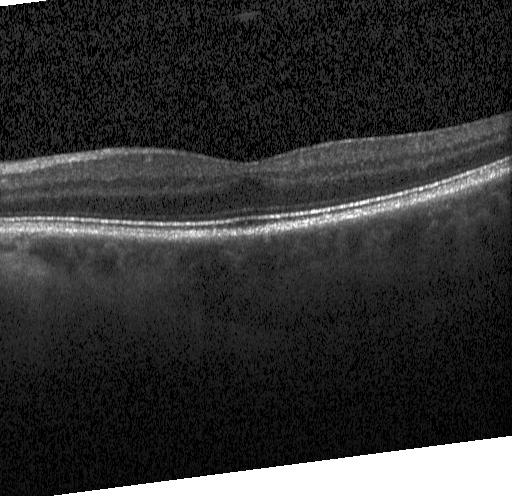

Dx: no choroidal neovascularization, diabetic macular edema, or drusen.